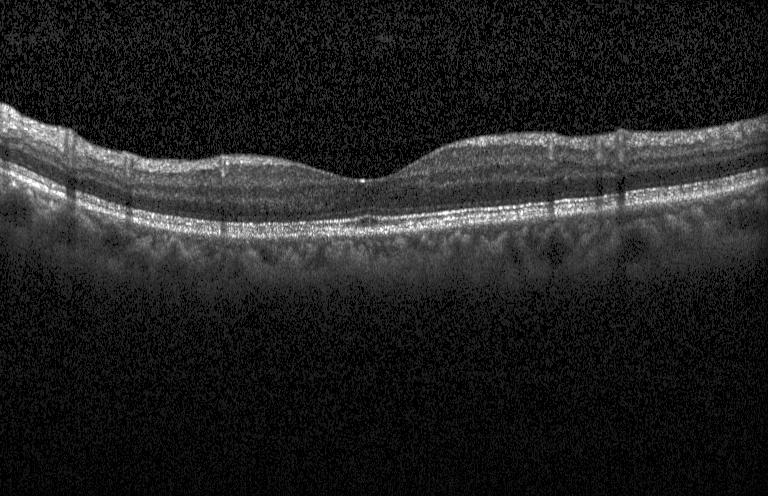
OCT line scan.
Impression: no CNV, no DME, and no drusen.